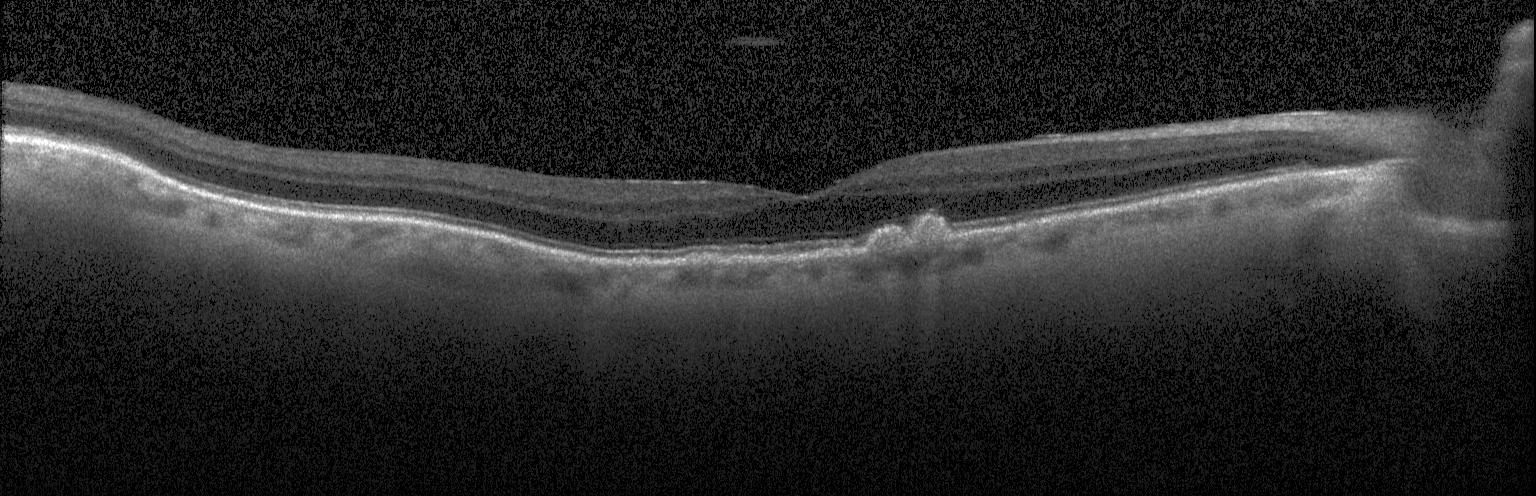 Assessment: multiple drusen.